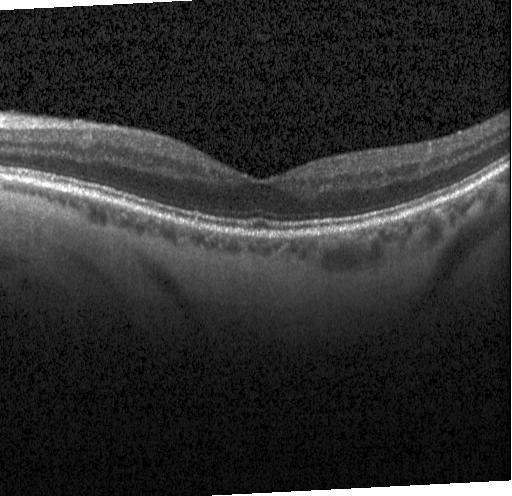

Instrument: Heidelberg Spectralis; spectral-domain optical coherence tomography; centered on the fovea; optical coherence tomography B-scan.
This B-scan demonstrates neither CNV, DME, nor drusen.